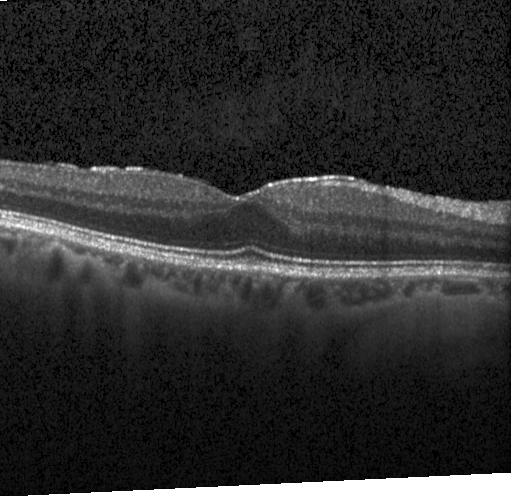 SD-OCT, acquired on a Heidelberg Spectralis, horizontal scan through the fovea, retinal OCT cross-section
Finding: no choroidal neovascularization, no diabetic macular edema, and no drusen.